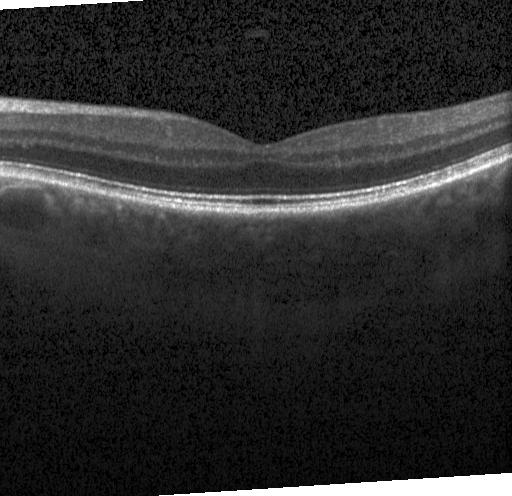 Horizontal scan through the fovea; SD-OCT; retinal OCT B-scan. Diagnosis: no evidence of CNV, DME, or drusen.